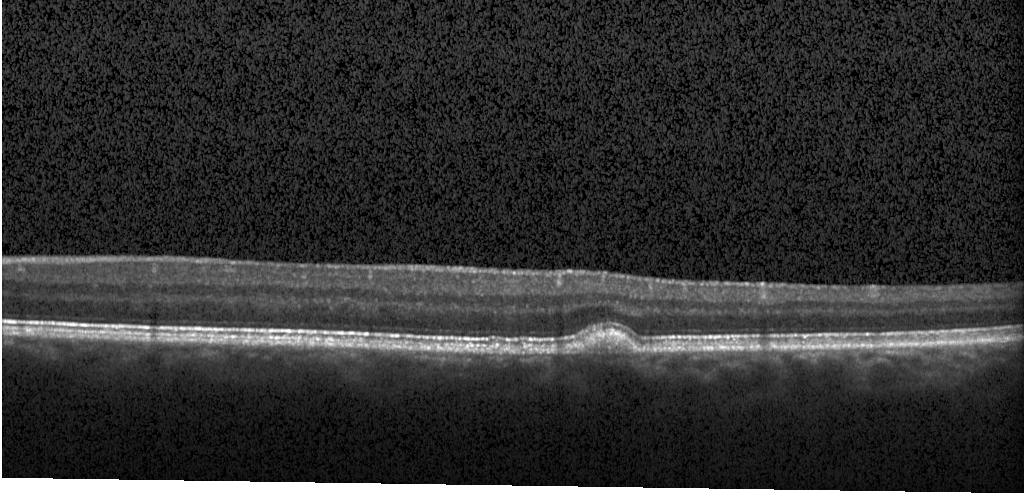

Impression: drusen.